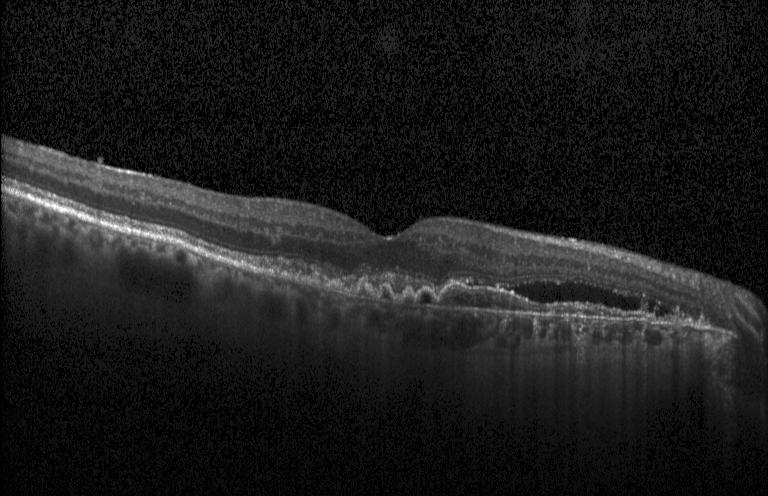

Through the macula · spectral-domain optical coherence tomography · Heidelberg Spectralis · retinal OCT cross-section. Finding: a choroidal neovascular membrane.